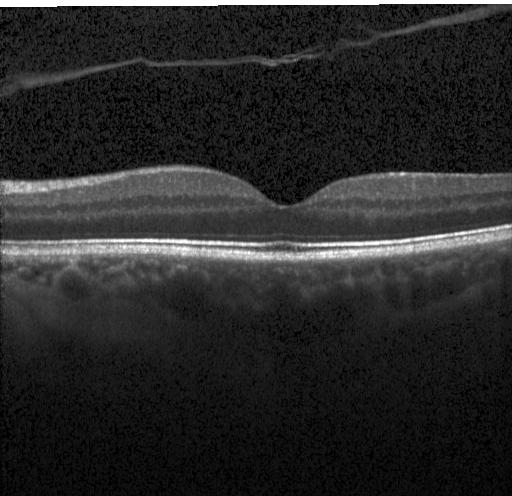

Assessment: neither choroidal neovascularization, diabetic macular edema, nor drusen.